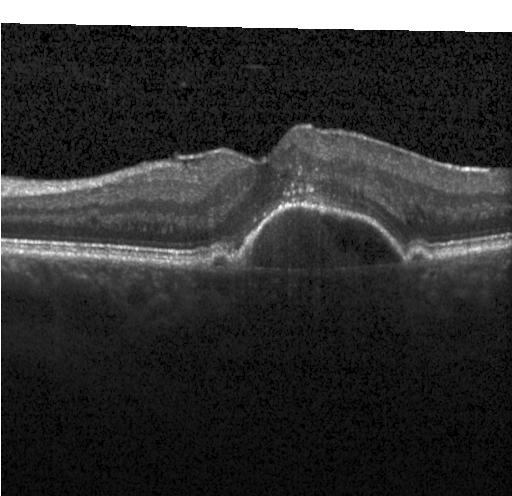

Spectral-domain optical coherence tomography. Retinal OCT cross-section.
Finding: a choroidal neovascular membrane.